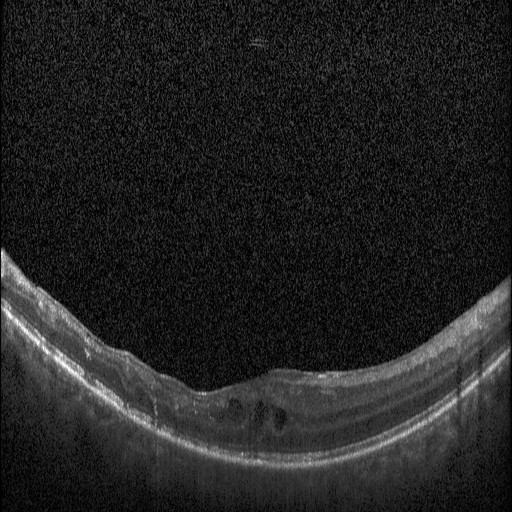 Optical coherence tomography B-scan. Spectral-domain optical coherence tomography. Through the macula
Diagnosis: DME.